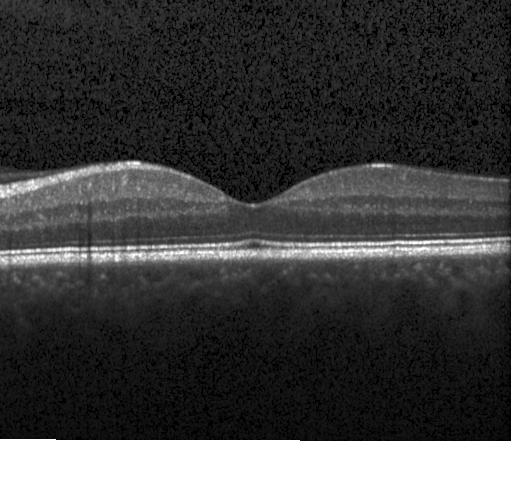 Diagnosis: no choroidal neovascularization, no diabetic macular edema, and no drusen.